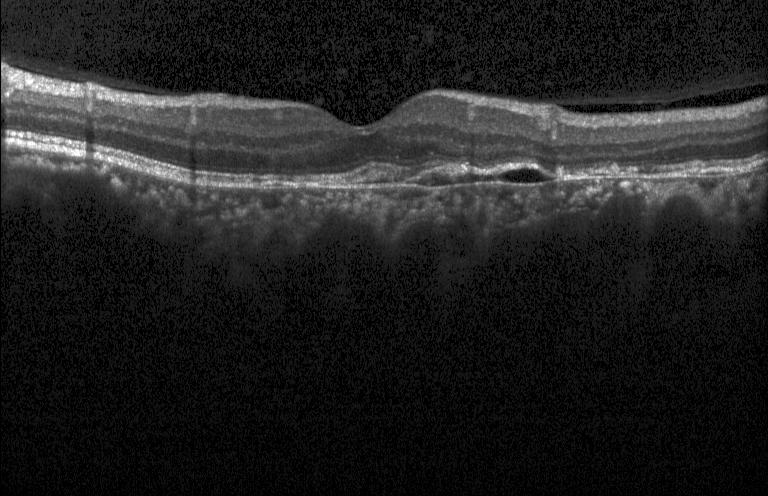 Spectral-domain OCT. Heidelberg Spectralis OCT system. Centered on the fovea. Retinal OCT B-scan. Impression: a choroidal neovascular membrane.